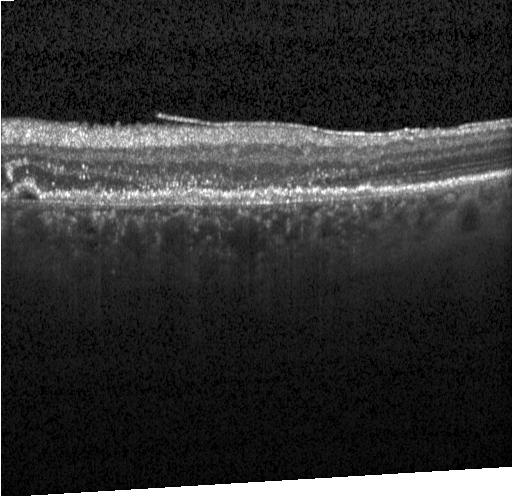 Heidelberg Spectralis OCT system; spectral-domain OCT; fovea-centered; optical coherence tomography scan. Assessment: choroidal neovascularization (CNV).